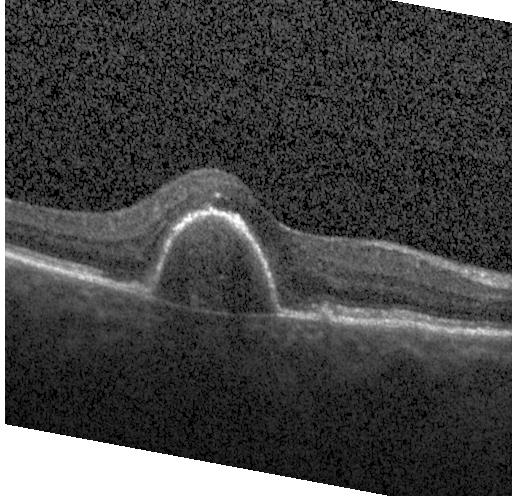
Retinal OCT cross-section.
Choroidal neovascularization (CNV).